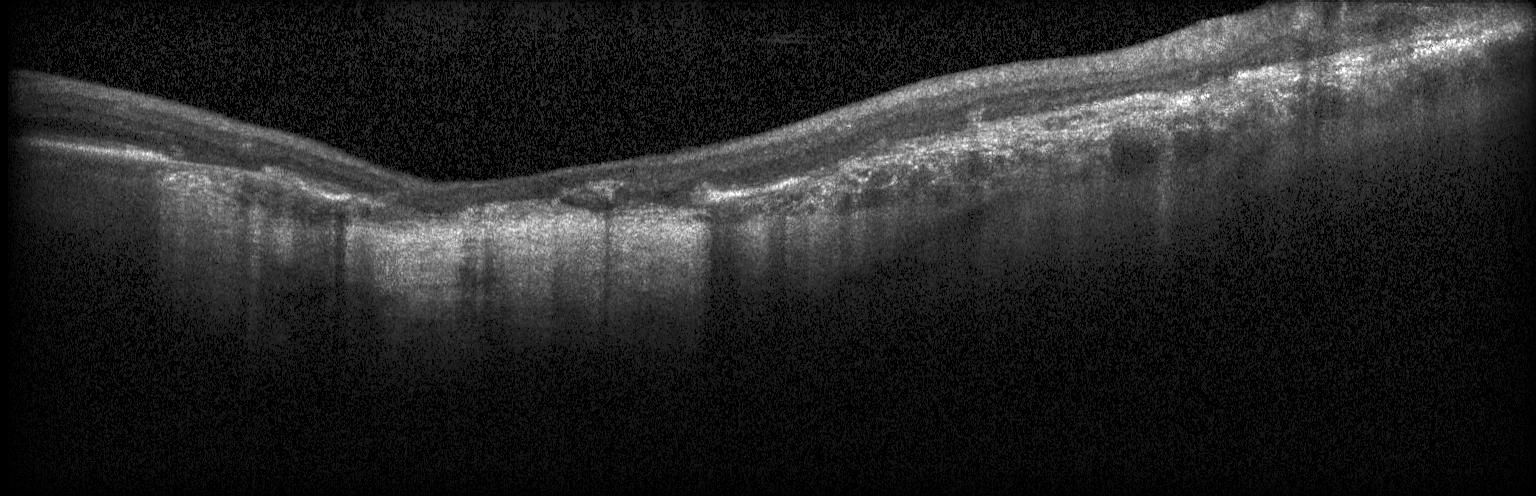

Fovea-centered · acquired on a Heidelberg Spectralis · SD-OCT · retinal OCT B-scan
This B-scan demonstrates choroidal neovascularization.